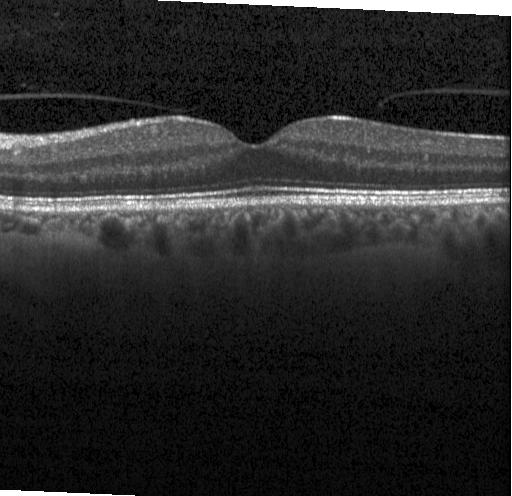
Centered on the fovea, spectral-domain optical coherence tomography, Heidelberg Spectralis, OCT B-scan. Assessment: no evidence of CNV, DME, or drusen.